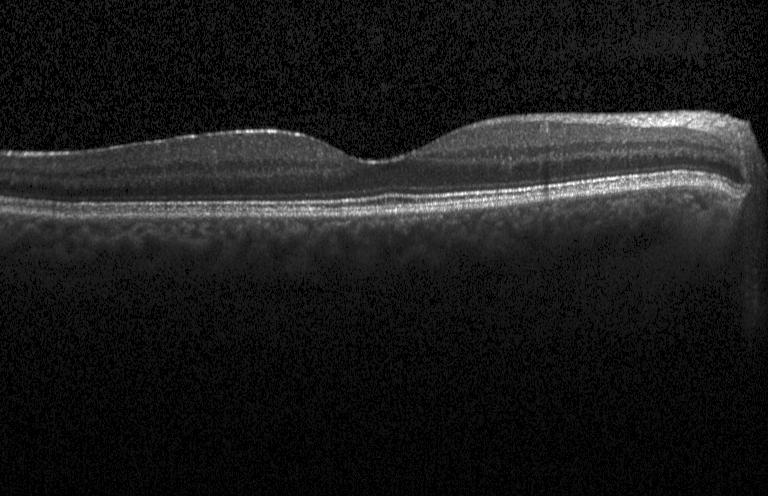
Impression: no evidence of choroidal neovascularization, diabetic macular edema, or drusen.